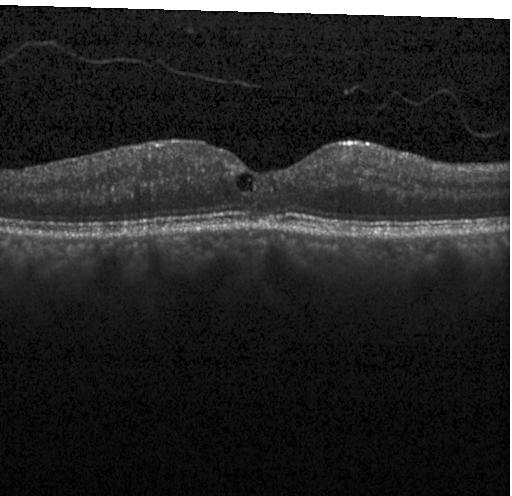

SD-OCT · Heidelberg Spectralis OCT system · optical coherence tomography scan · macular scan.
Finding: diabetic macular edema.